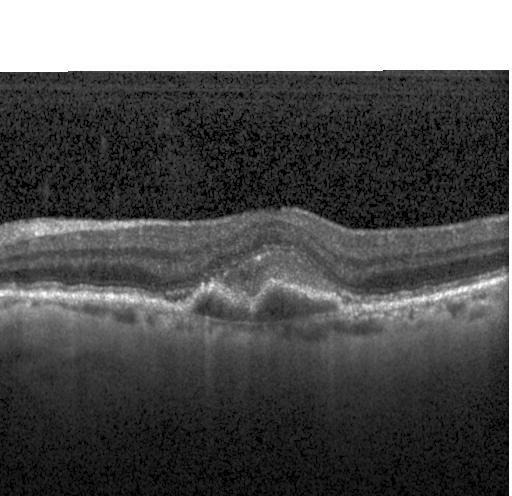 OCT B-scan. This B-scan demonstrates a choroidal neovascular membrane.